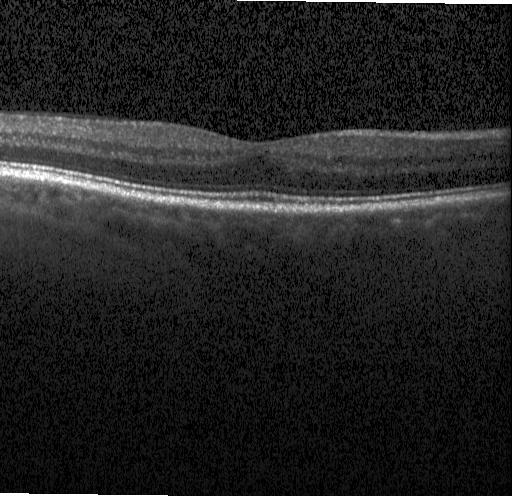 No choroidal neovascularization, no diabetic macular edema, and no drusen.